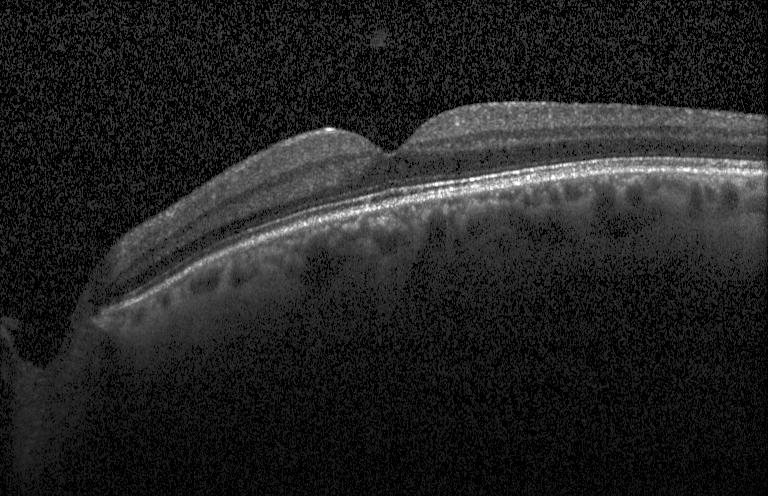
Centered on the fovea, spectral-domain OCT, optical coherence tomography B-scan — The scan shows neither CNV, DME, nor drusen.